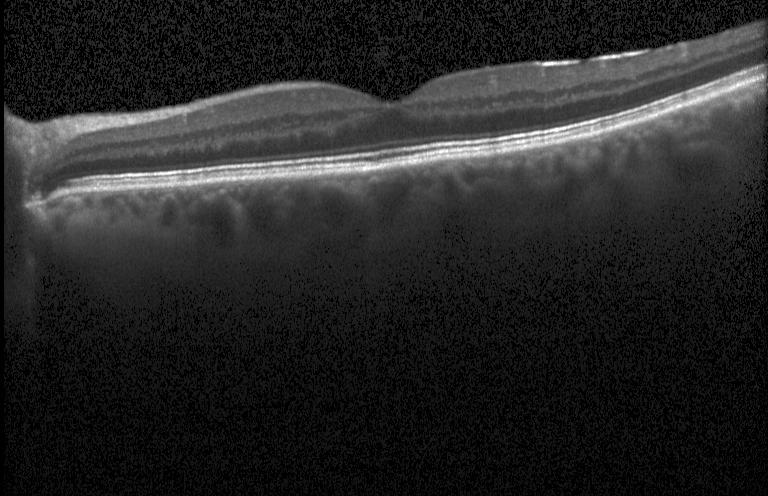
Retinal OCT B-scan — Impression: no evidence of CNV, DME, or drusen.